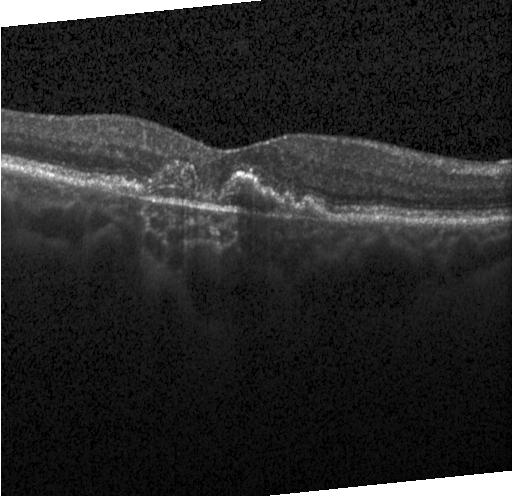

OCT line scan, macular scan, Heidelberg Spectralis OCT system, SD-OCT — Impression: a choroidal neovascular membrane.